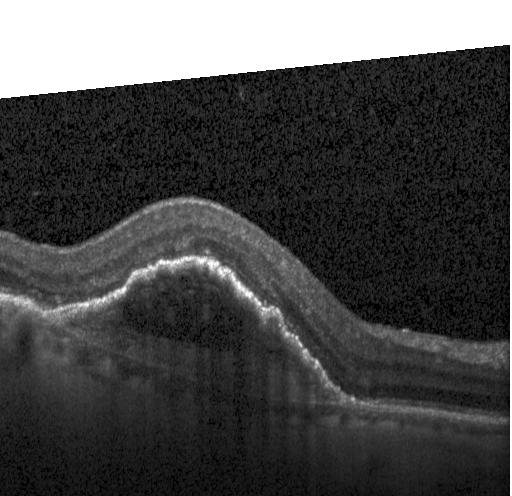
Macular OCT demonstrating choroidal neovascularization.